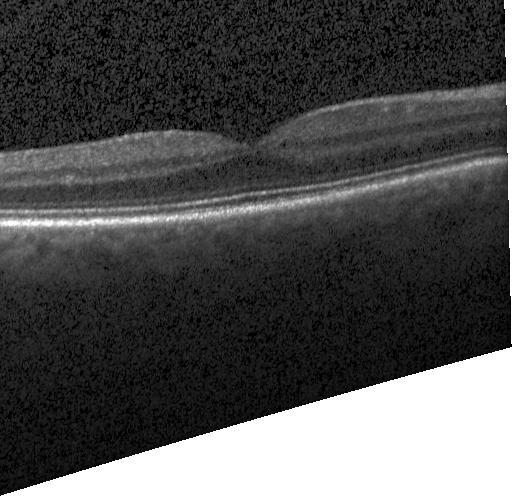

OCT line scan
Assessment: neither choroidal neovascularization, diabetic macular edema, nor drusen.